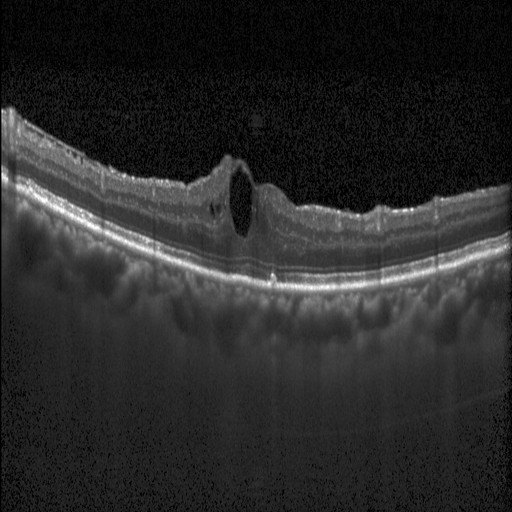
Impression: diabetic macular edema.